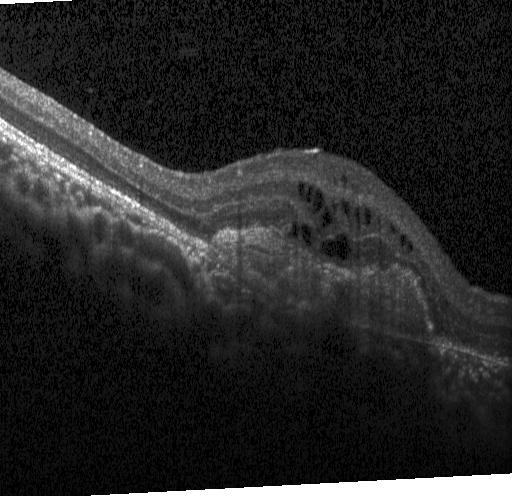 Heidelberg Spectralis; spectral-domain OCT; macular scan; OCT line scan
Dx: a choroidal neovascular membrane.